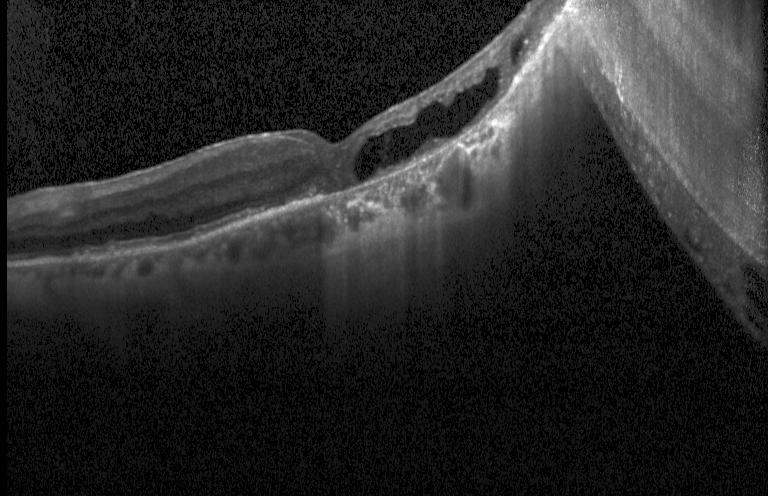 The scan shows diabetic macular edema (DME).